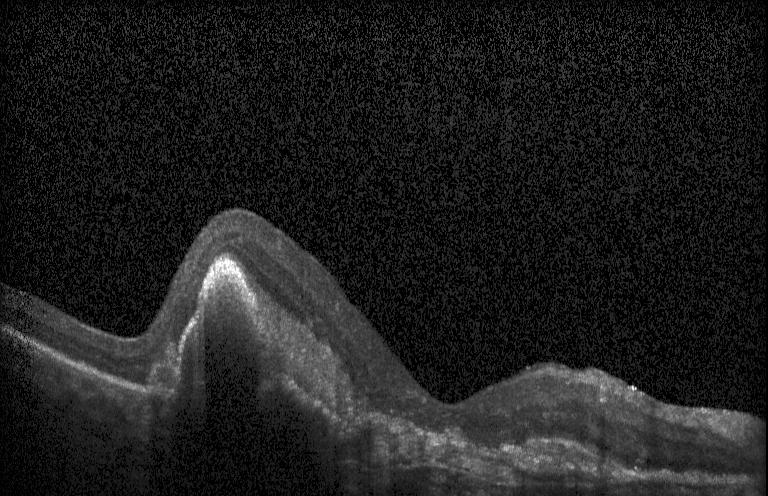 Retinal OCT cross-section. Acquired on a Heidelberg Spectralis. Finding: choroidal neovascularization.